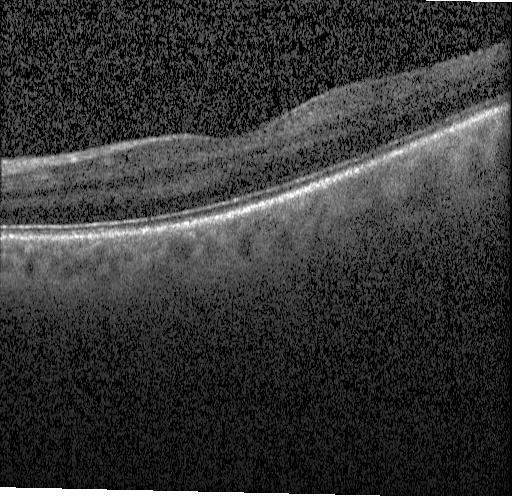 Retinal OCT B-scan.
Diagnosis: no CNV, DME, or drusen.